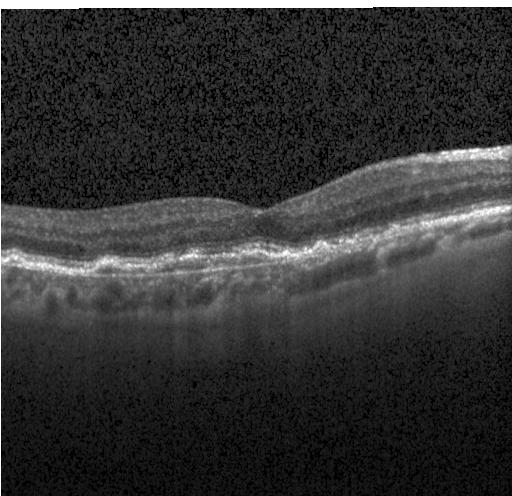
Dx: a choroidal neovascular membrane.